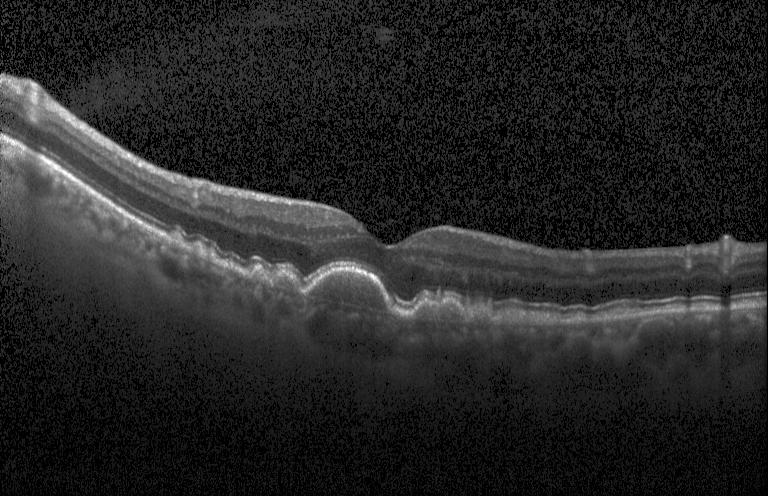 Optical coherence tomography B-scan.
Assessment: drusen.